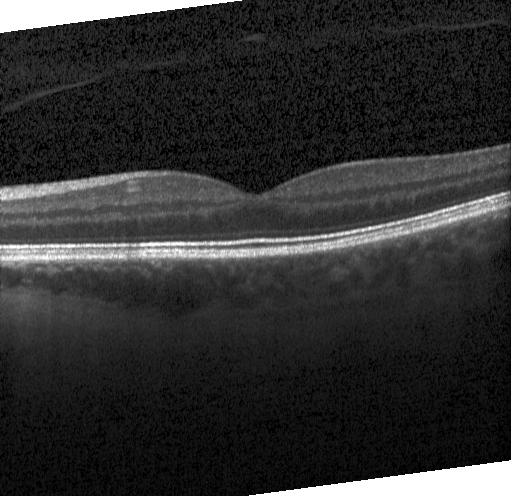
Centered on the fovea, retinal OCT B-scan, SD-OCT, Heidelberg Spectralis OCT system.
No choroidal neovascularization, no diabetic macular edema, and no drusen.